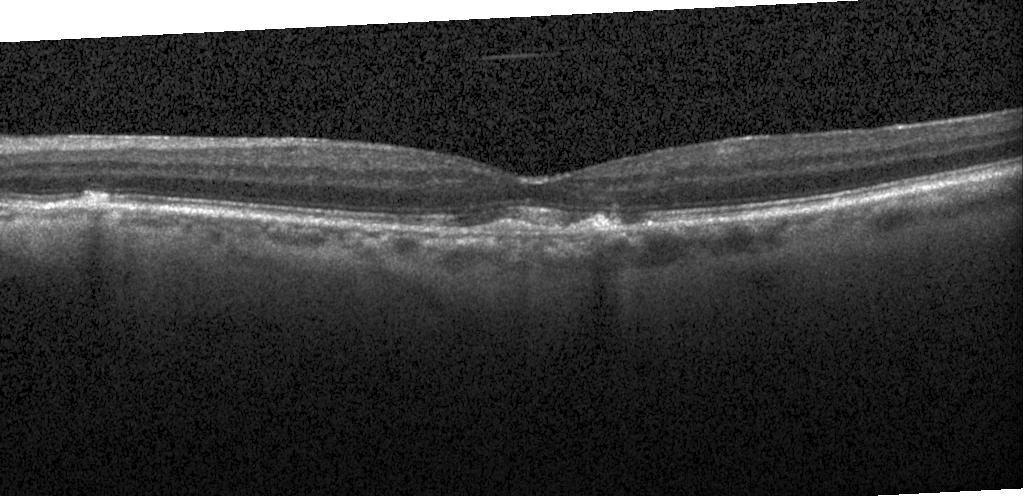 Retinal OCT B-scan
Diagnosis: CNV.